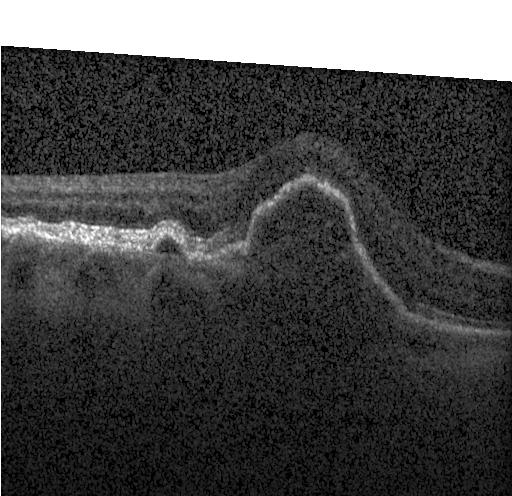 This B-scan demonstrates a choroidal neovascular membrane.